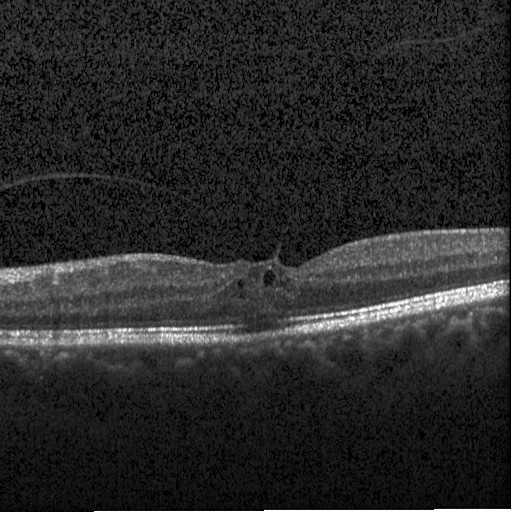
Spectral-domain OCT B-scan: diabetic macular edema.